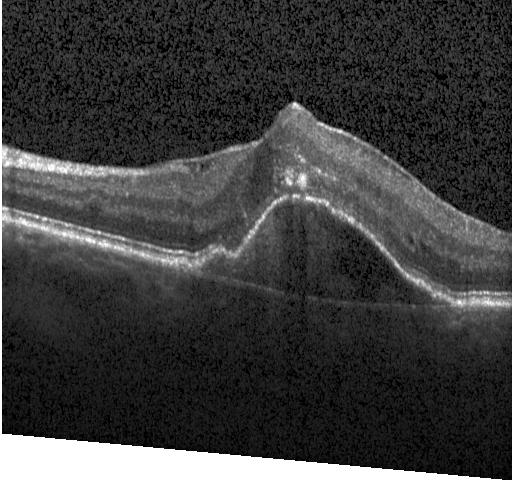

Fovea-centered; retinal OCT B-scan; spectral-domain OCT; instrument: Heidelberg Spectralis.
Impression: a choroidal neovascular membrane.